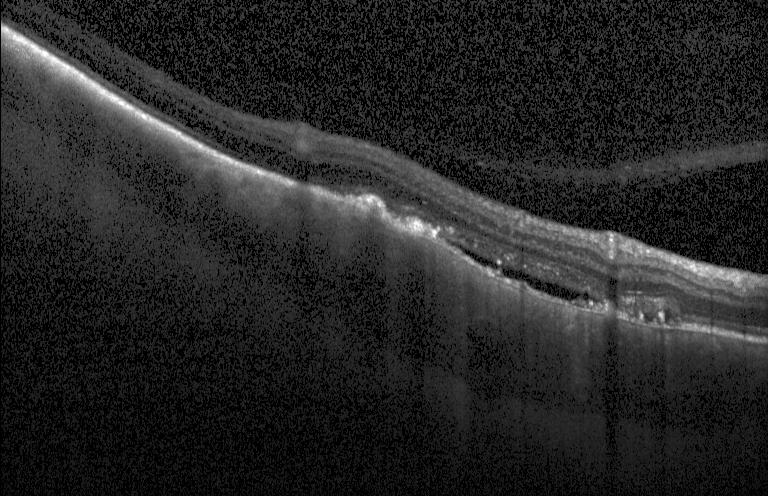 OCT B-scan; SD-OCT
Impression: a choroidal neovascular membrane.